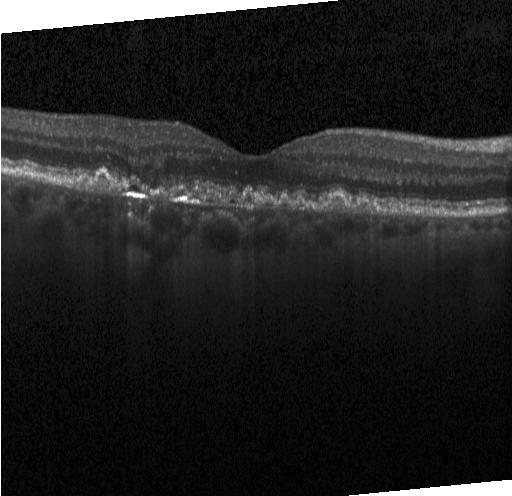 SD-OCT; optical coherence tomography scan.
OCT finding: choroidal neovascularization (CNV).